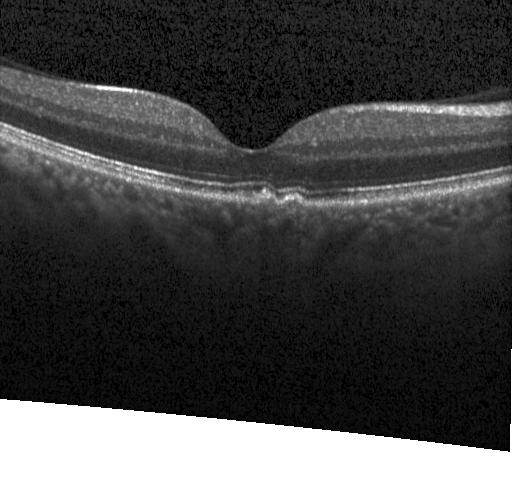 Impression: sub-RPE drusenoid deposits.